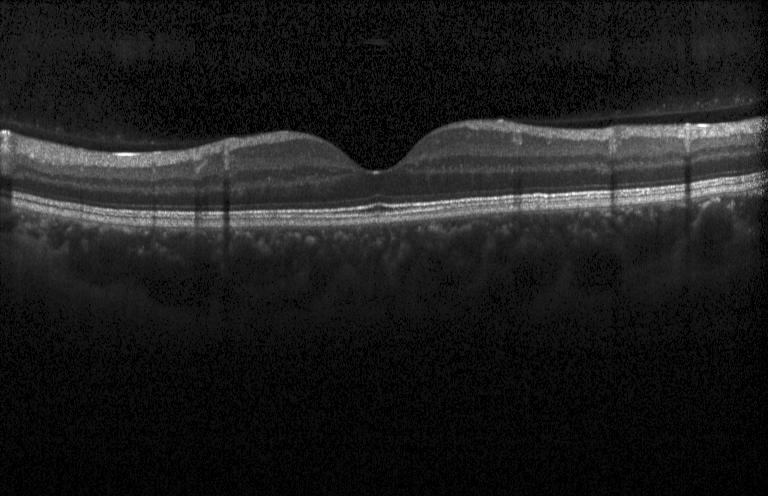
Heidelberg Spectralis; OCT line scan. OCT finding: neither CNV, DME, nor drusen.